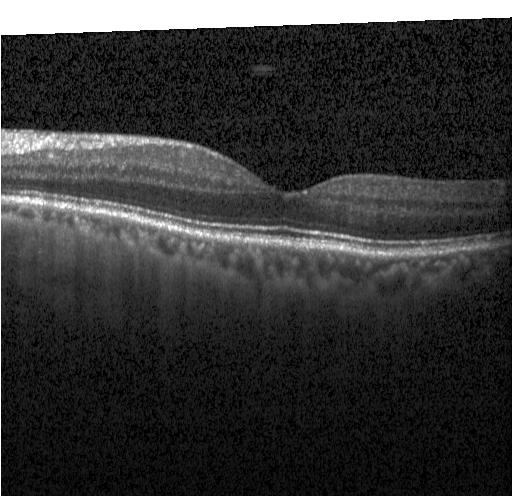 SD-OCT, through the macula, optical coherence tomography B-scan, Heidelberg Spectralis OCT system — Impression: no choroidal neovascularization, no diabetic macular edema, and no drusen.